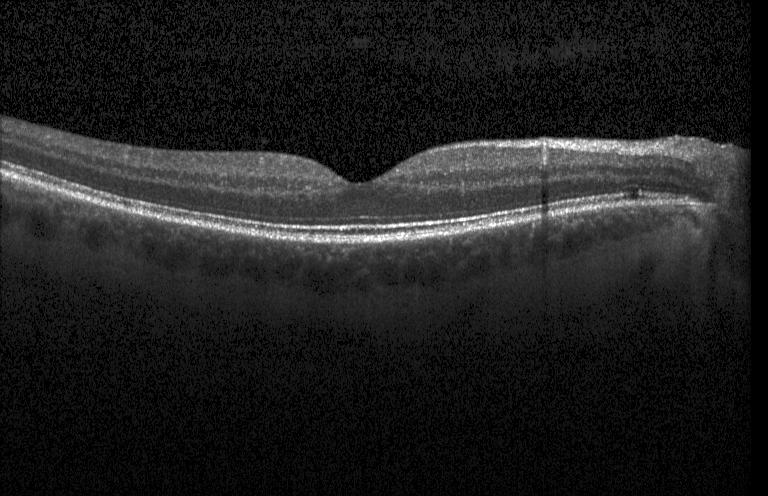
Optical coherence tomography scan. Heidelberg Spectralis. Spectral-domain OCT. Fovea-centered. No choroidal neovascularization, diabetic macular edema, or drusen.